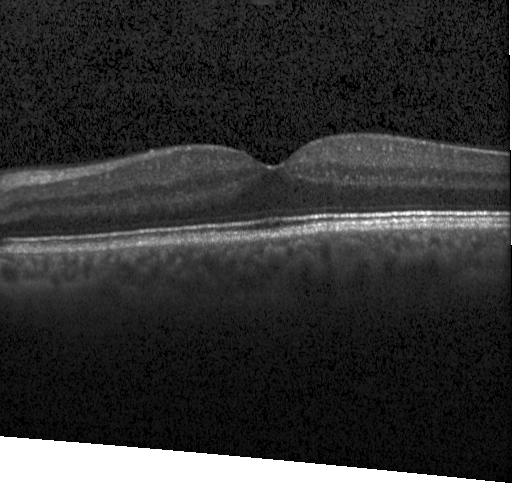 Retinal OCT cross-section showing no evidence of choroidal neovascularization, diabetic macular edema, or drusen.